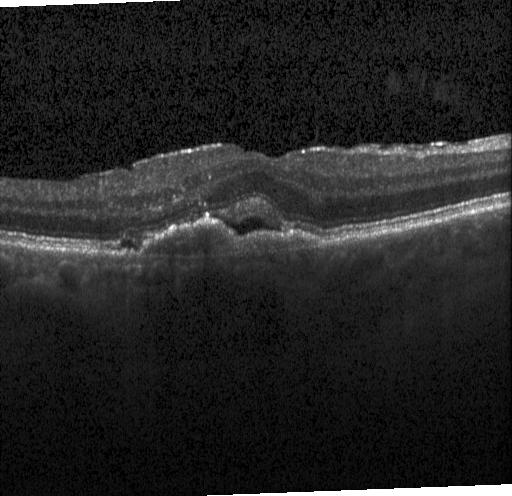 Through the macula. Optical coherence tomography scan. Spectral-domain optical coherence tomography.
Dx: a choroidal neovascular membrane.